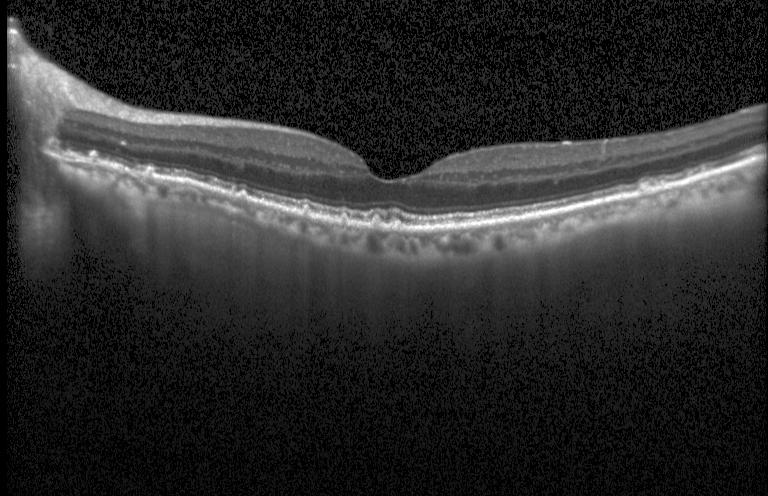 OCT finding: sub-RPE drusenoid deposits.